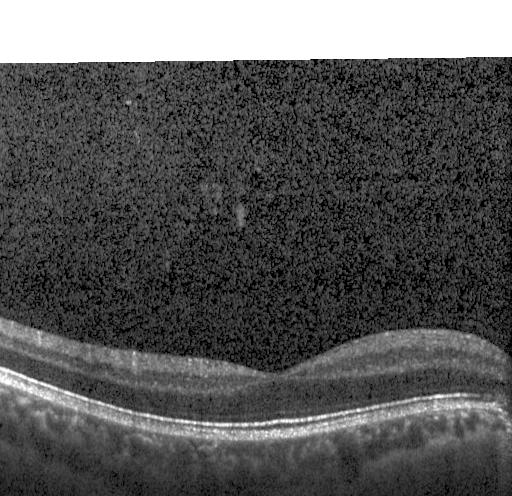

OCT line scan. Dx: neither choroidal neovascularization, diabetic macular edema, nor drusen.